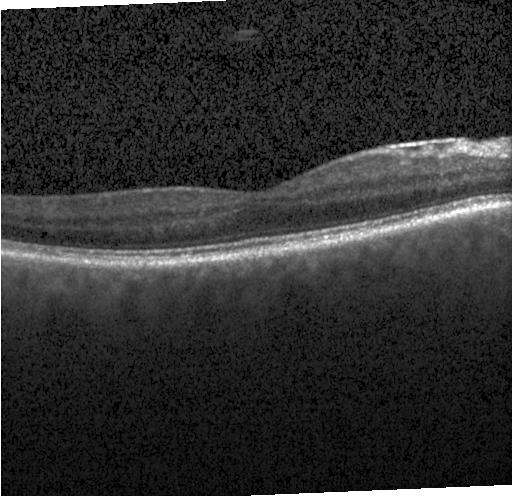 Dx: no CNV, DME, or drusen.